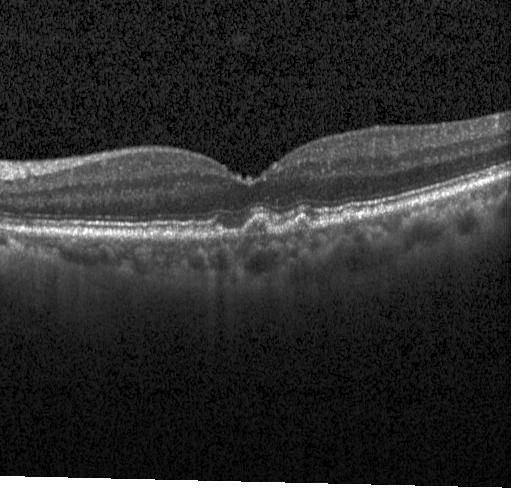 Macular OCT demonstrating drusen.